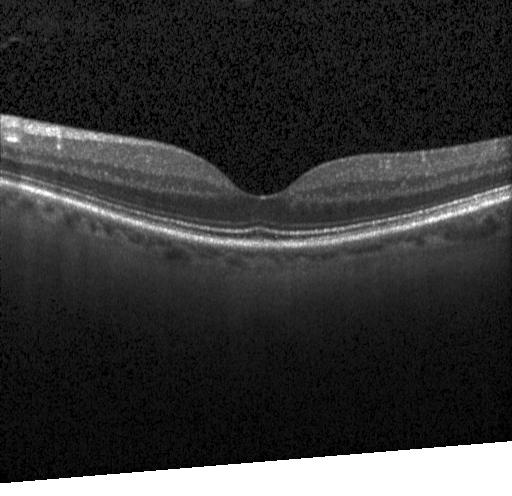

Dx: neither CNV, DME, nor drusen.